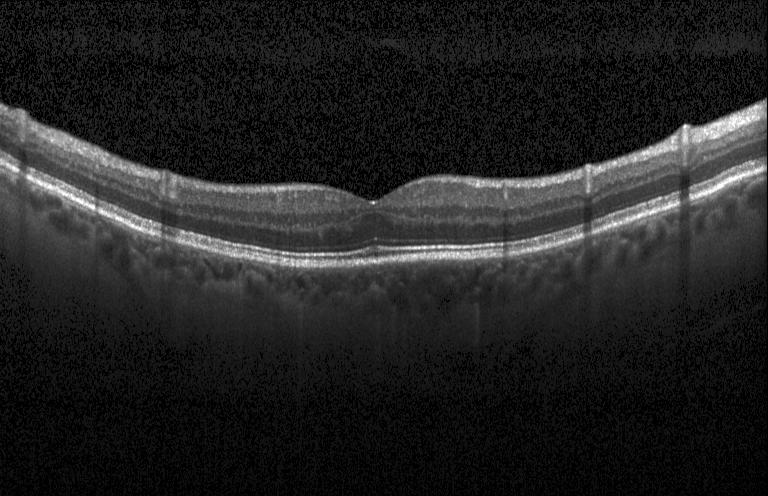 Retinal OCT cross-section — The scan shows neither choroidal neovascularization, diabetic macular edema, nor drusen.